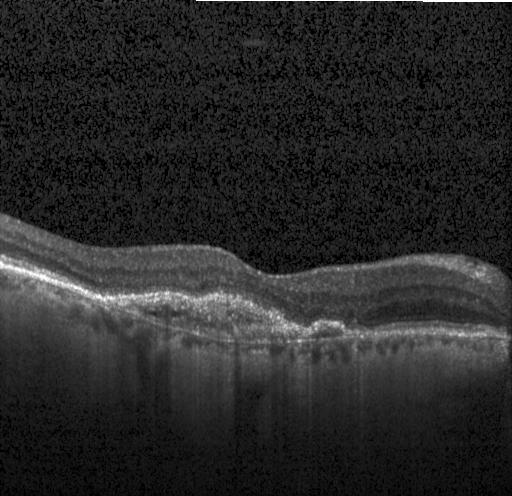

Optical coherence tomography B-scan
The scan shows a choroidal neovascular membrane.